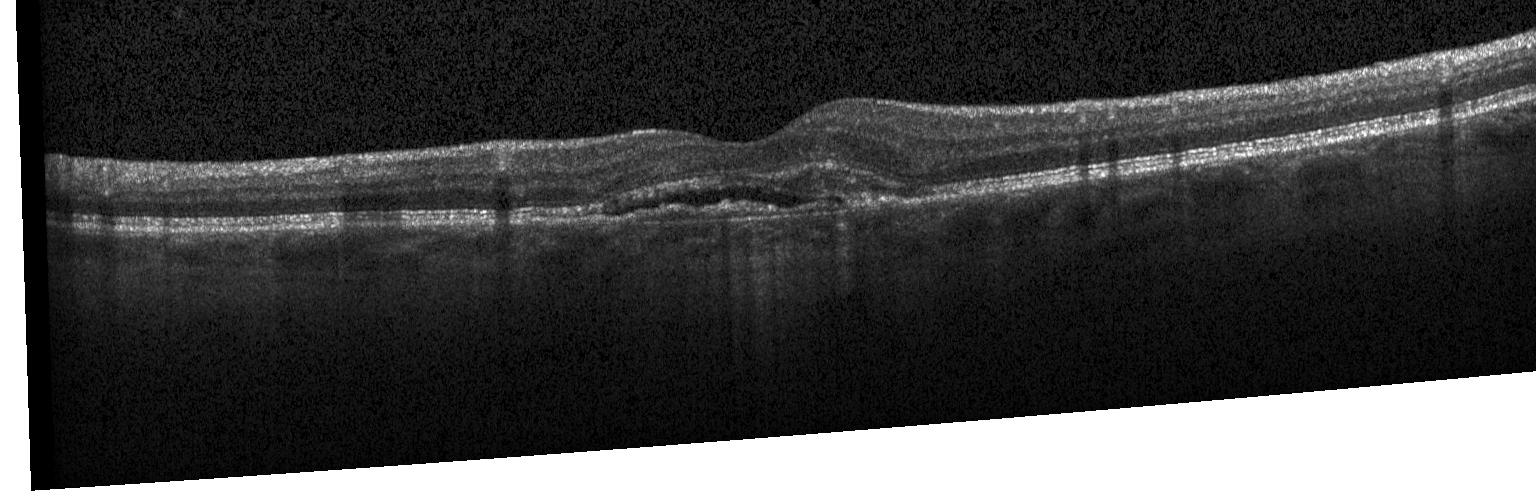 OCT line scan. Heidelberg Spectralis OCT system. SD-OCT — Assessment: a choroidal neovascular membrane.